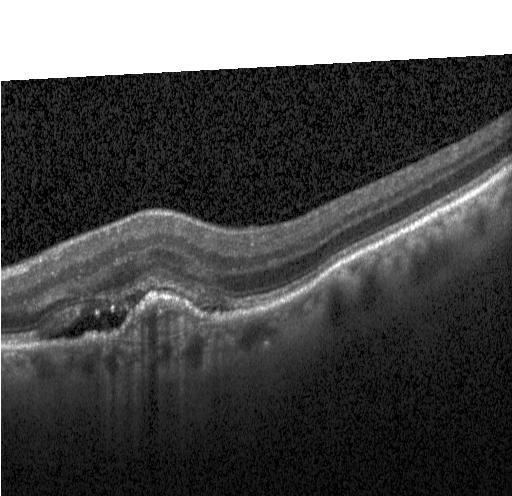

Spectral-domain OCT · horizontal scan through the fovea · optical coherence tomography B-scan
Choroidal neovascularization (CNV).